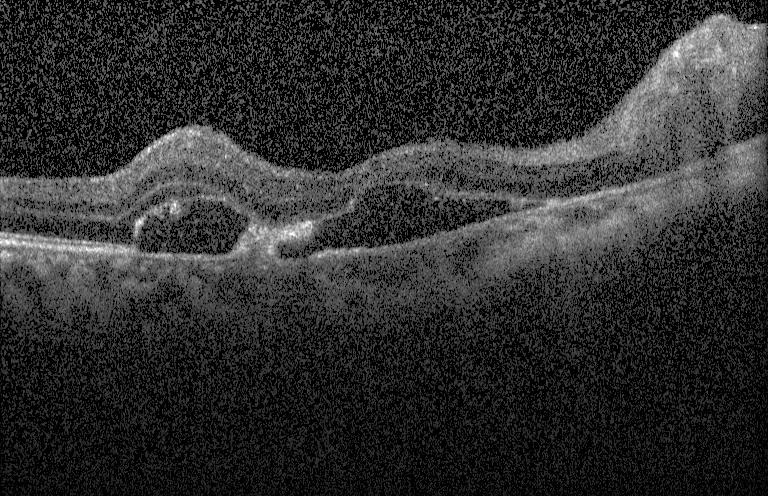

Retinal OCT cross-section showing a choroidal neovascular membrane.